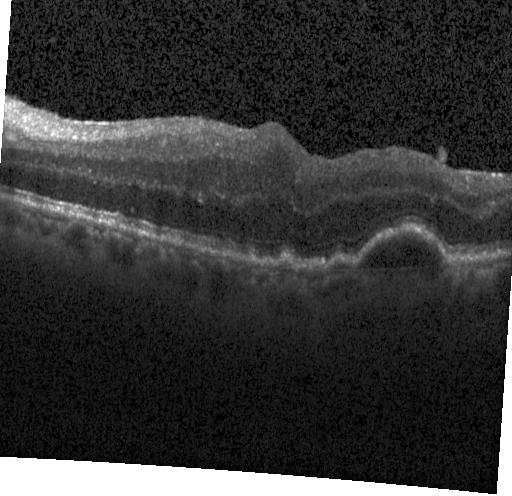
Optical coherence tomography B-scan, macular scan, spectral-domain optical coherence tomography, acquired on a Heidelberg Spectralis. Diagnosis: a choroidal neovascular membrane.